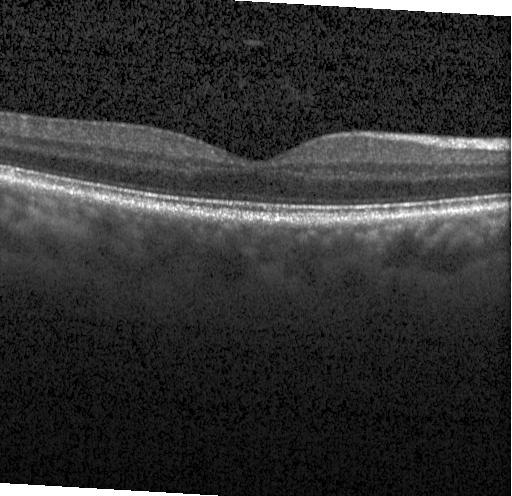

Macular OCT: neither choroidal neovascularization, diabetic macular edema, nor drusen.